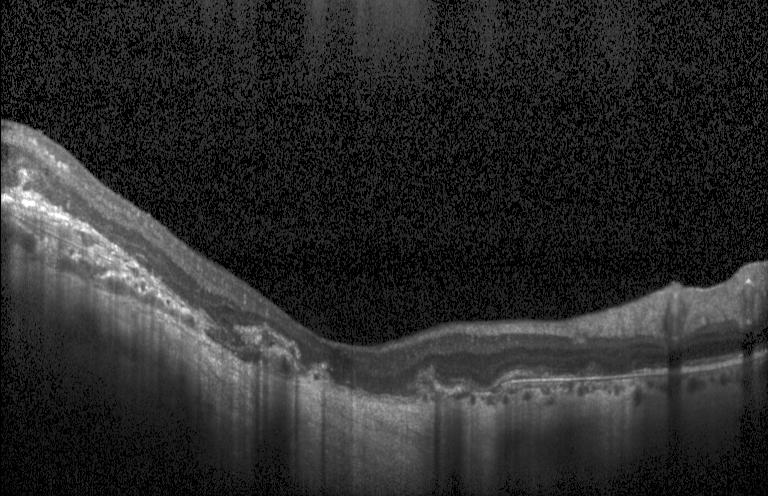

Optical coherence tomography scan.
Assessment: choroidal neovascularization (CNV).